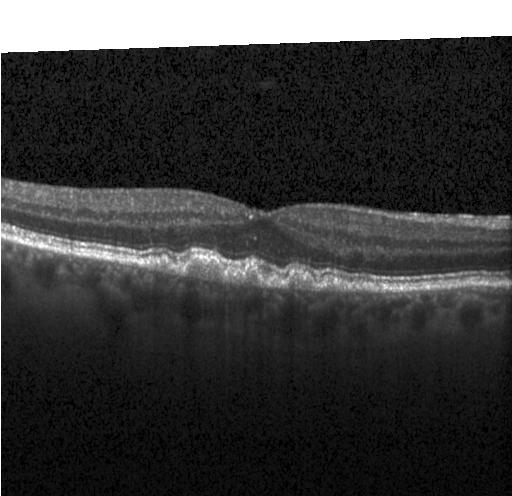 Macular scan; Heidelberg Spectralis; retinal OCT cross-section — This B-scan demonstrates sub-RPE drusenoid deposits.